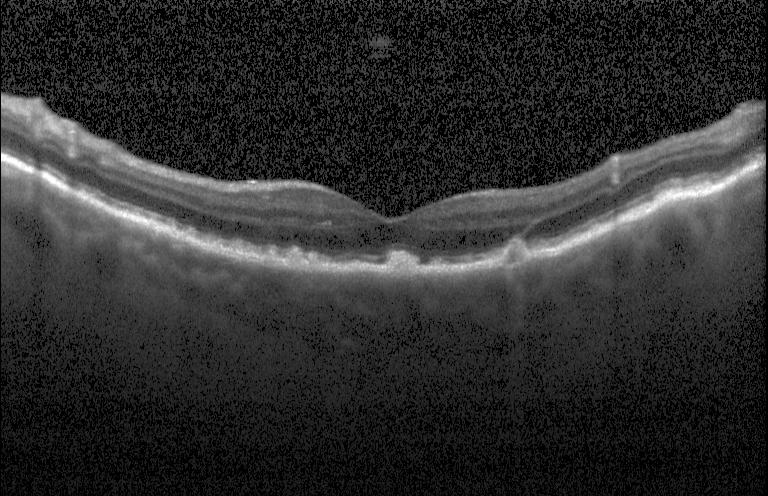 Finding: a choroidal neovascular membrane.